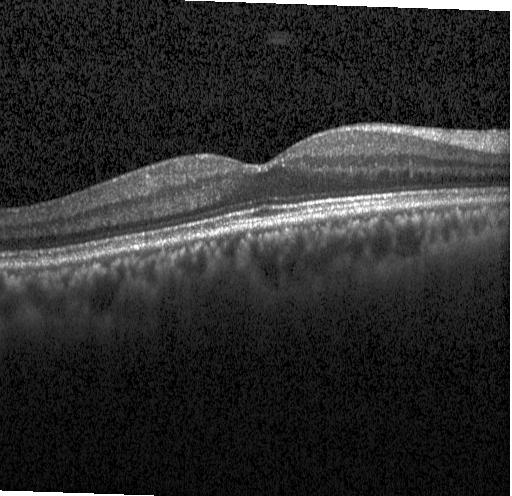

Impression: no evidence of choroidal neovascularization, diabetic macular edema, or drusen.